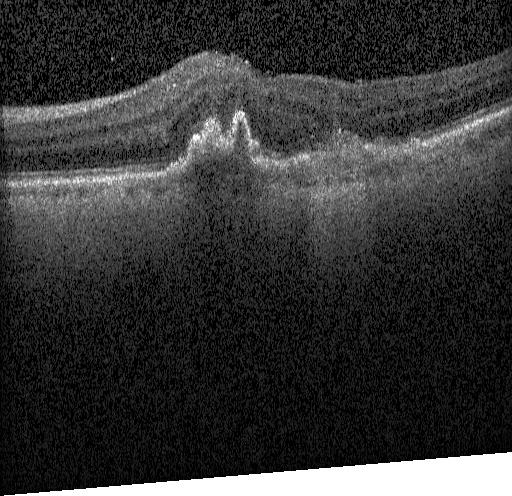
Macular scan · optical coherence tomography scan
OCT finding: a choroidal neovascular membrane.